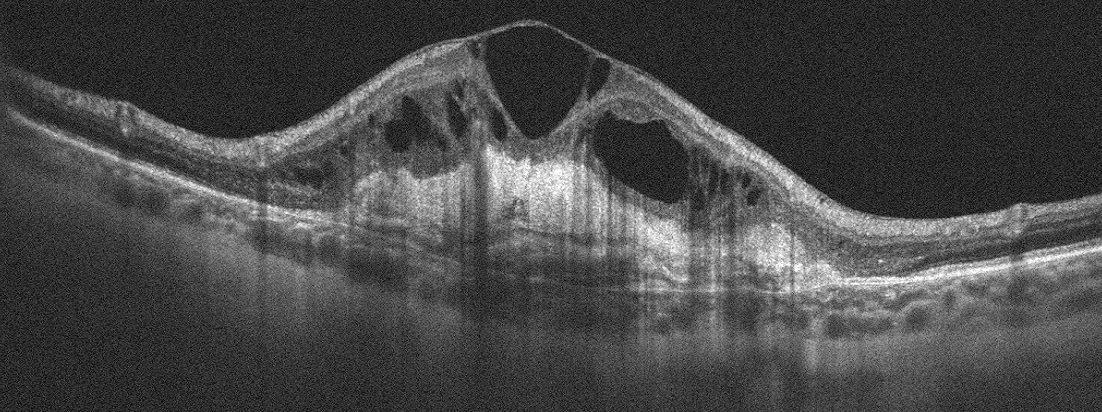
Finding: age-related macular degeneration (AMD).